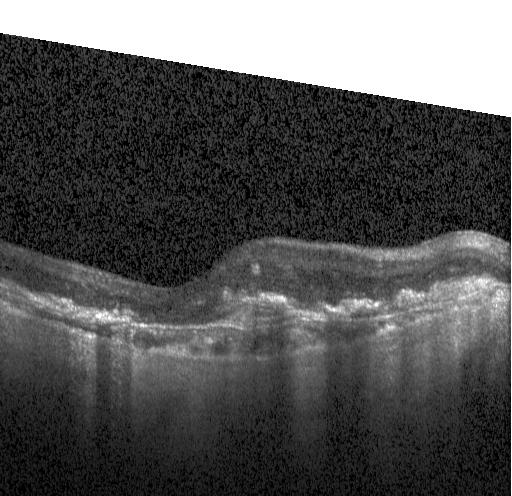
Spectral-domain optical coherence tomography · optical coherence tomography B-scan · acquired on a Heidelberg Spectralis
Macular OCT: a choroidal neovascular membrane.